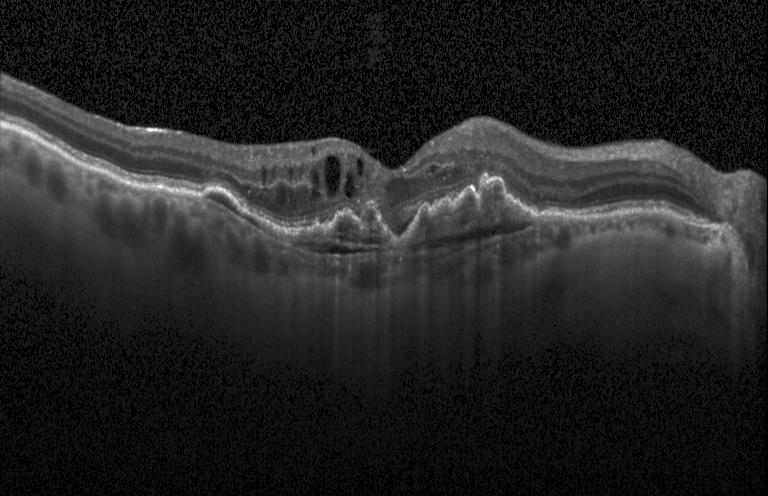 Fovea-centered; retinal OCT B-scan; Heidelberg Spectralis; SD-OCT. Finding: a choroidal neovascular membrane.